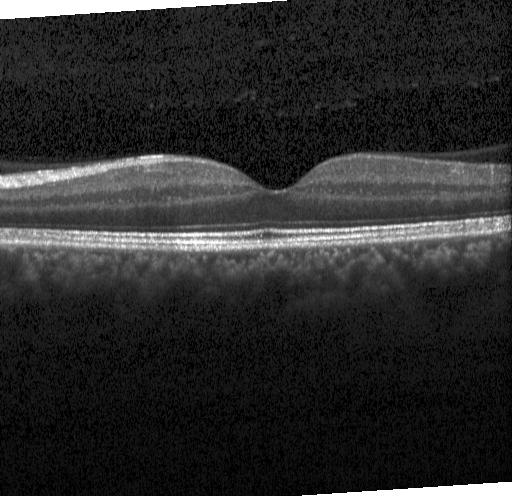

Heidelberg Spectralis · optical coherence tomography B-scan. Assessment: no choroidal neovascularization, diabetic macular edema, or drusen.